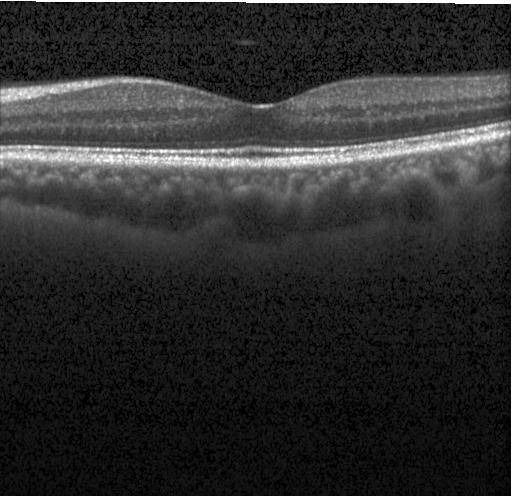 Optical coherence tomography B-scan — Finding: no CNV, DME, or drusen.